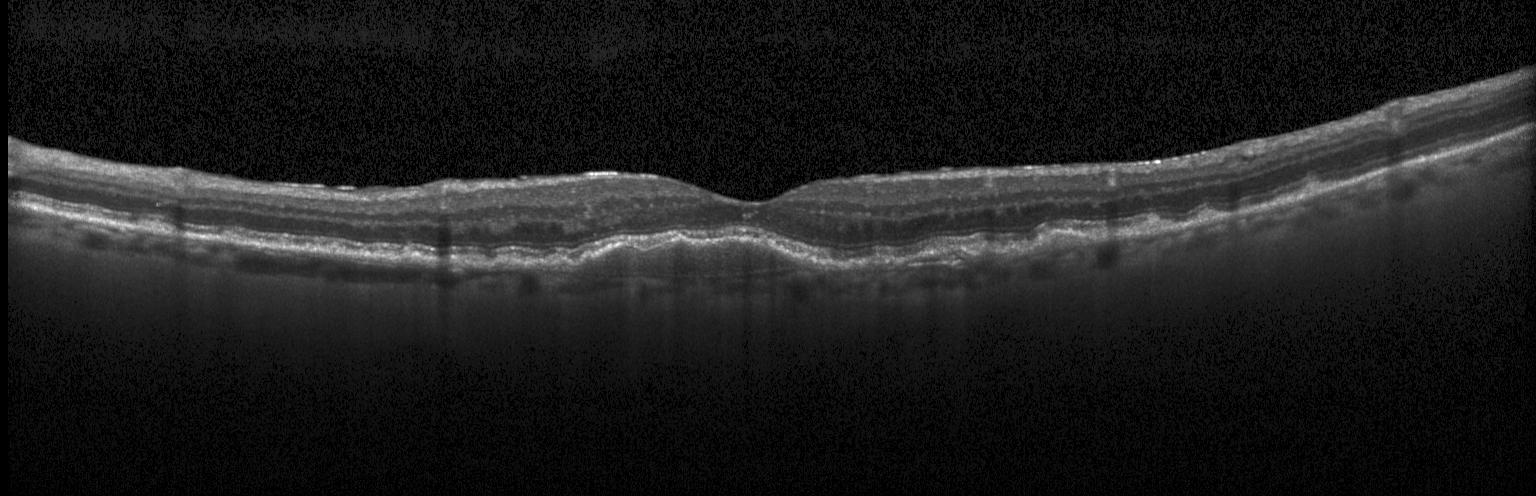 Macular OCT: a choroidal neovascular membrane.